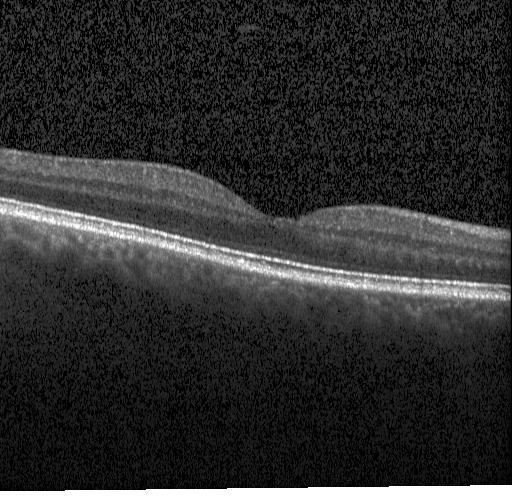

Fovea-centered · OCT B-scan · Heidelberg Spectralis — Diagnosis: no evidence of choroidal neovascularization, diabetic macular edema, or drusen.